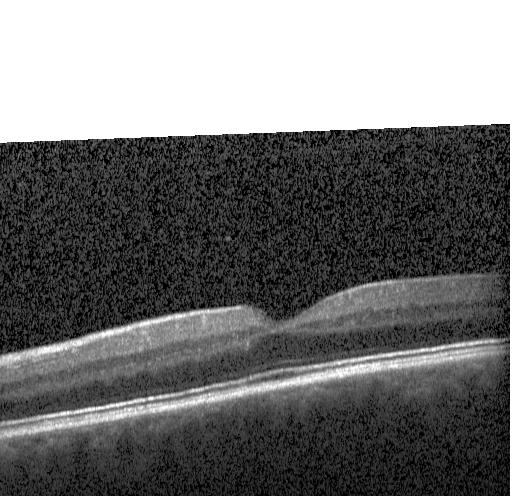 Spectral-domain optical coherence tomography, retinal OCT B-scan, fovea-centered — Diagnosis: no choroidal neovascularization, no diabetic macular edema, and no drusen.